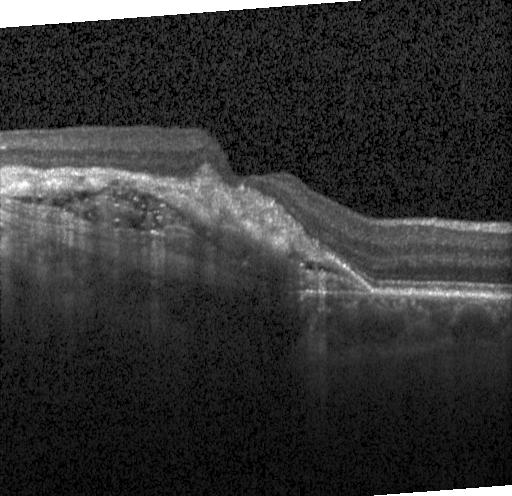
Dx: CNV.